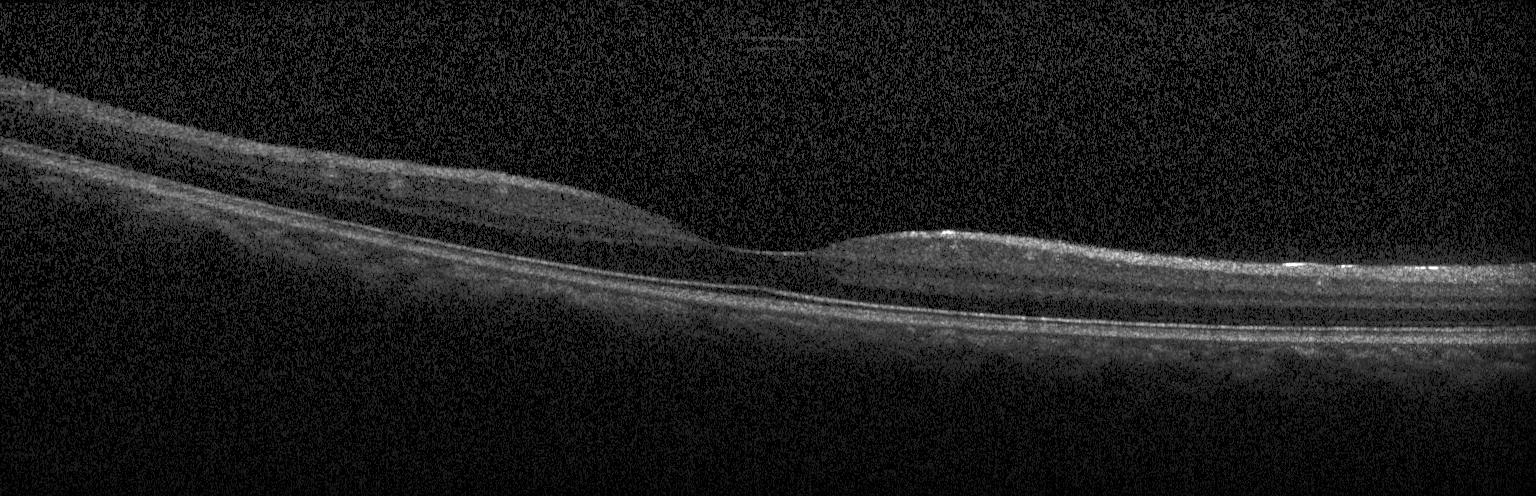 Impression: no choroidal neovascularization, diabetic macular edema, or drusen.